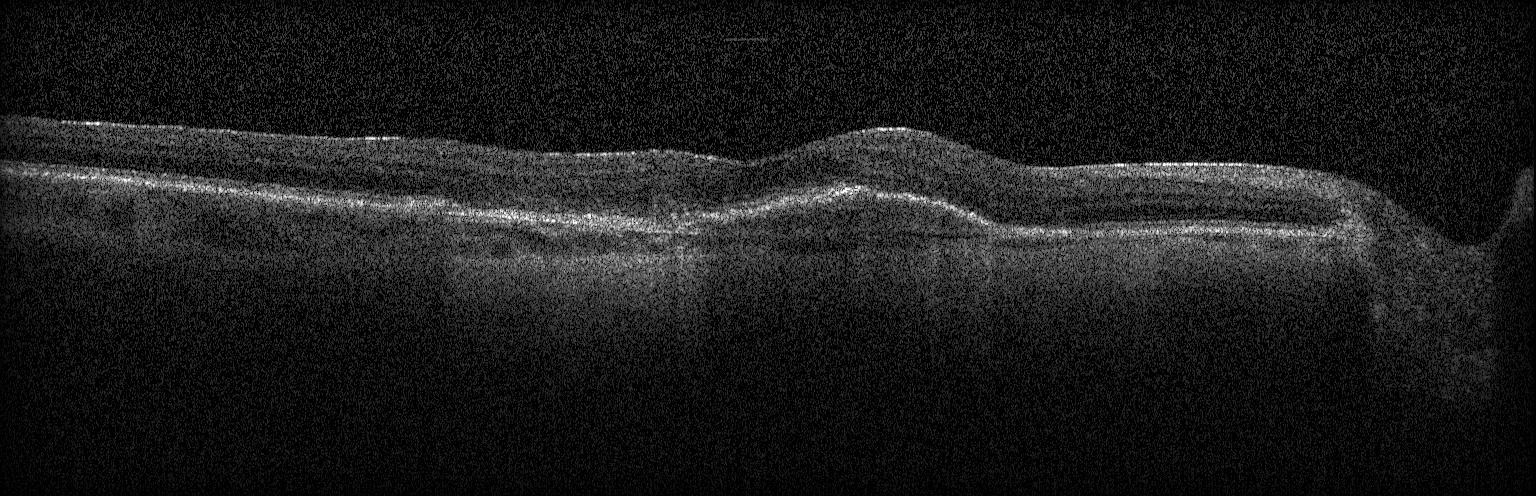
Dx: CNV.